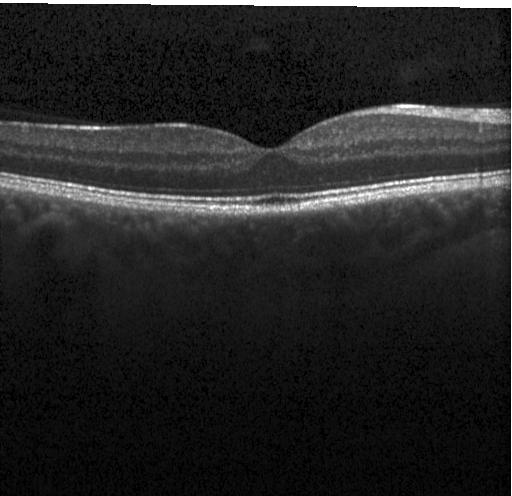

Retinal OCT B-scan, acquired on a Heidelberg Spectralis, SD-OCT, centered on the fovea.
Macular OCT: no choroidal neovascularization, no diabetic macular edema, and no drusen.